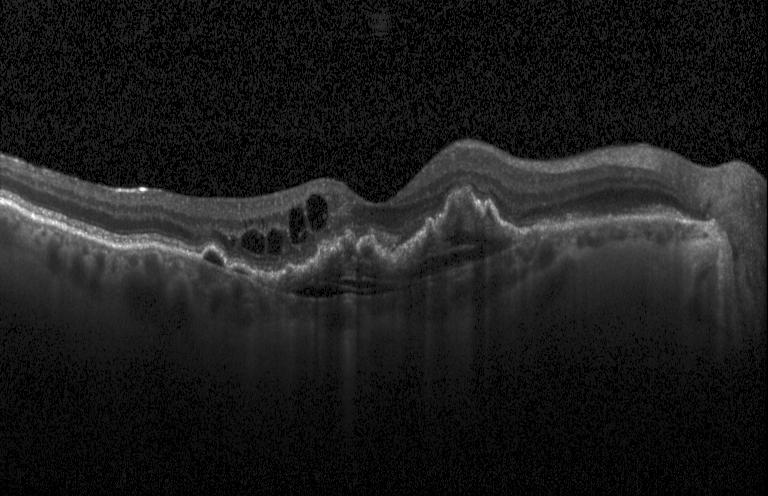
OCT B-scan showing choroidal neovascularization.